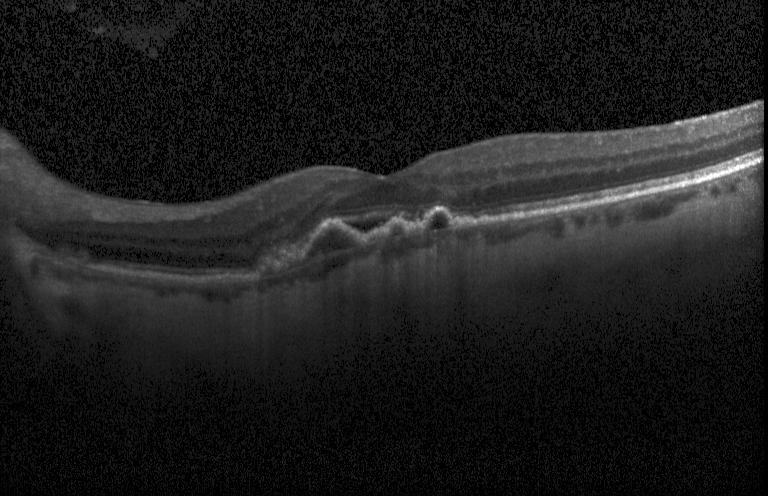 SD-OCT. Heidelberg Spectralis. Optical coherence tomography B-scan — Diagnosis: choroidal neovascularization.